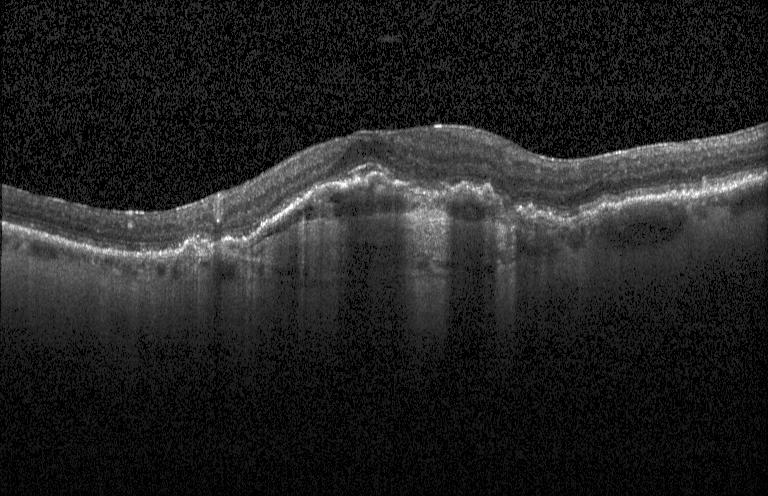 Macular scan; retinal OCT B-scan — The scan shows a choroidal neovascular membrane.